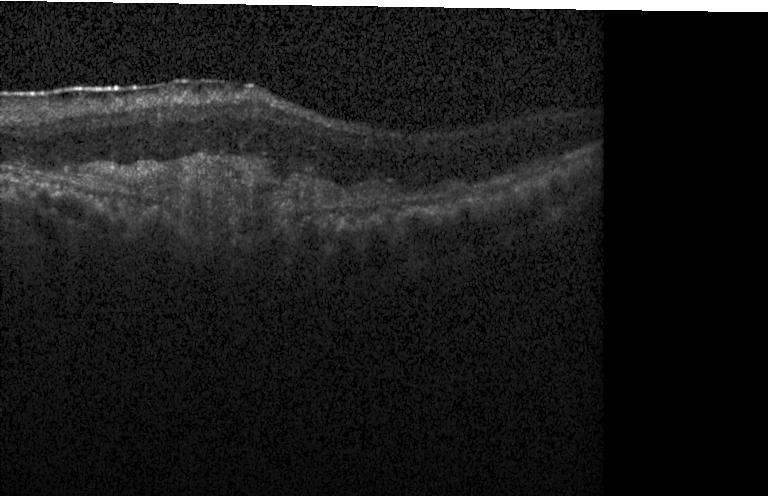 OCT line scan.
Finding: a choroidal neovascular membrane.